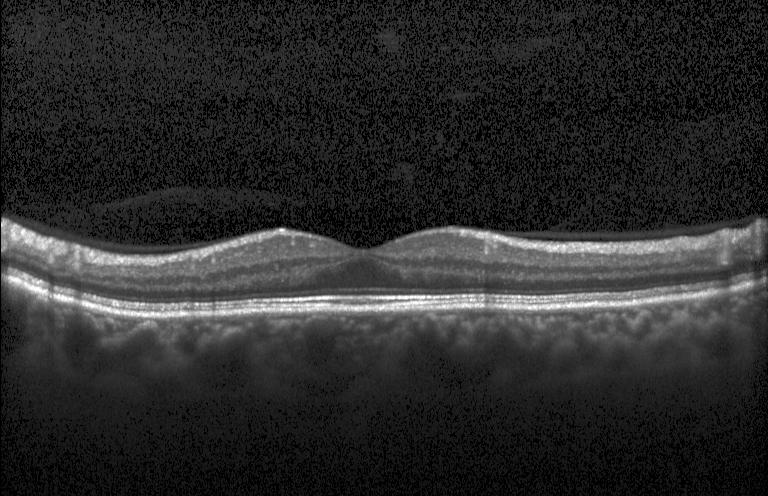
Centered on the fovea; SD-OCT; OCT line scan.
Diagnosis: no evidence of choroidal neovascularization, diabetic macular edema, or drusen.